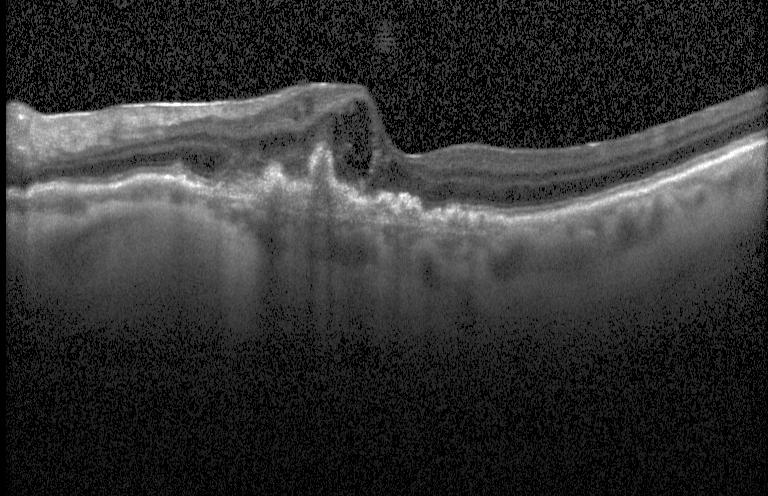

Optical coherence tomography scan. Heidelberg Spectralis — Diagnosis: a choroidal neovascular membrane.